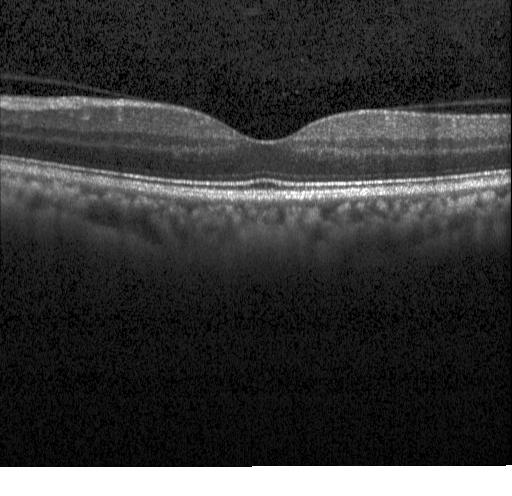 Optical coherence tomography B-scan.
This B-scan demonstrates no evidence of CNV, DME, or drusen.